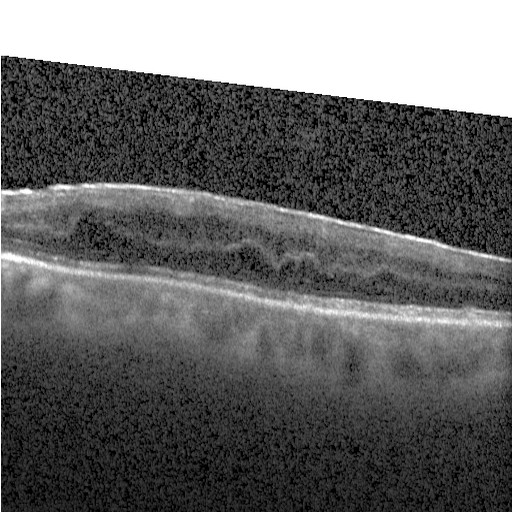 Macular OCT: diabetic macular edema (DME).